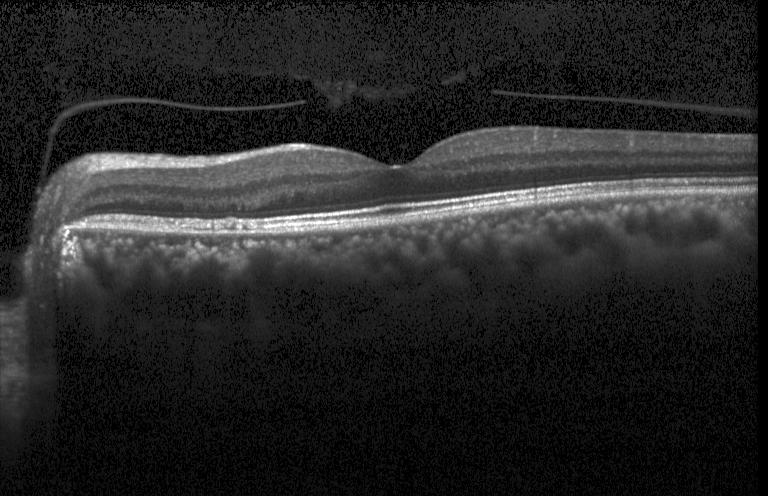

The scan shows neither choroidal neovascularization, diabetic macular edema, nor drusen.